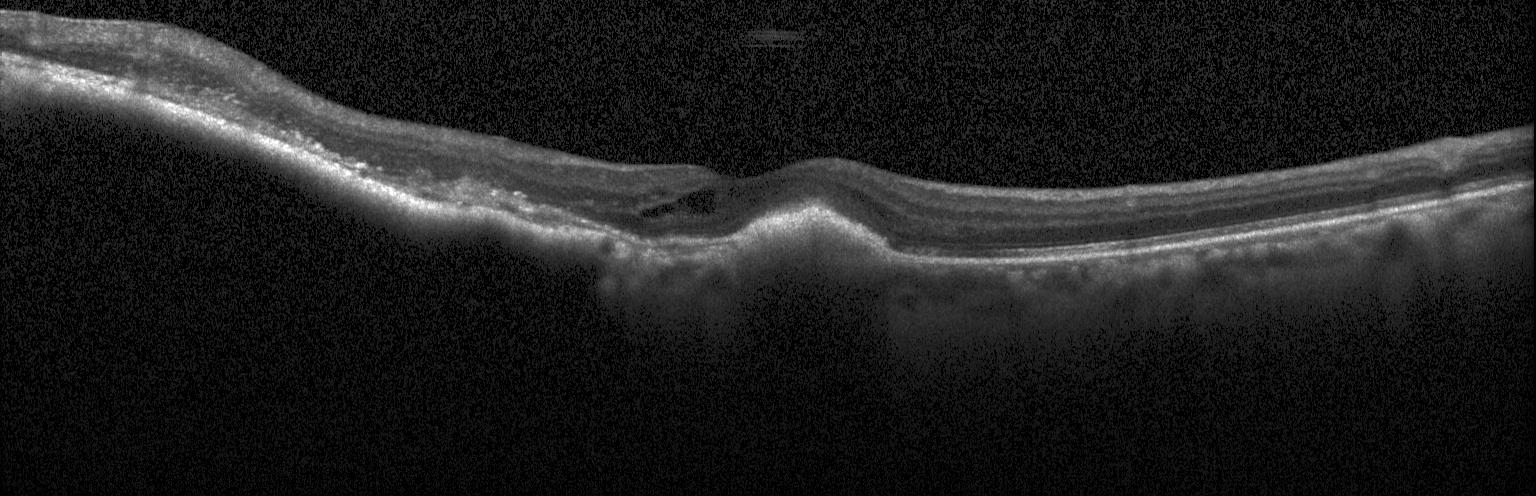 Spectral-domain OCT. Macular scan. Optical coherence tomography B-scan.
Impression: choroidal neovascularization.